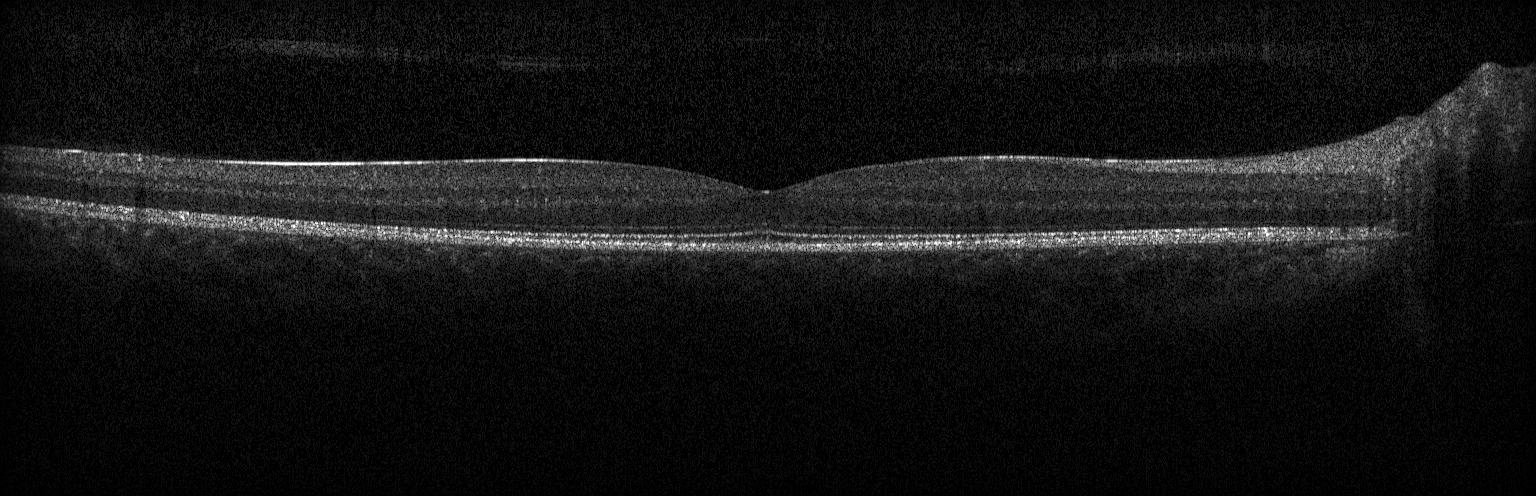 Macular OCT: no choroidal neovascularization, diabetic macular edema, or drusen.